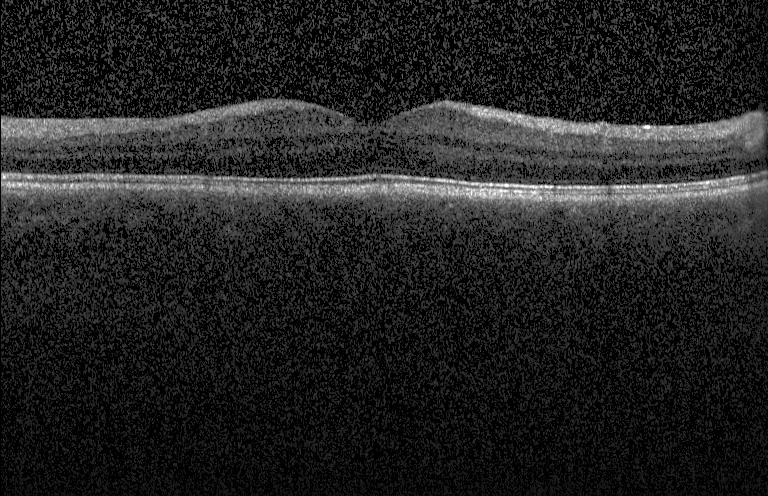
Macular OCT demonstrating neither choroidal neovascularization, diabetic macular edema, nor drusen.